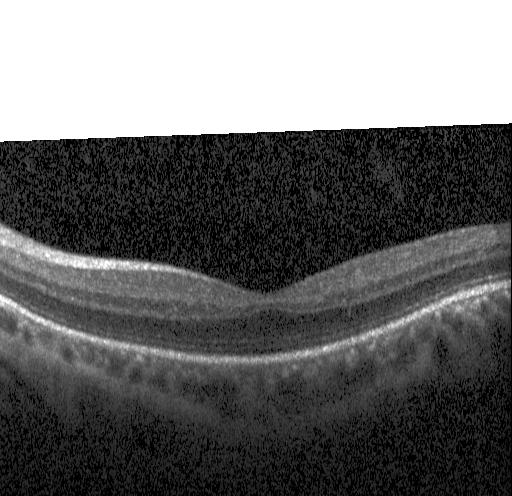

Through the macula; SD-OCT; retinal OCT B-scan.
Impression: no evidence of CNV, DME, or drusen.